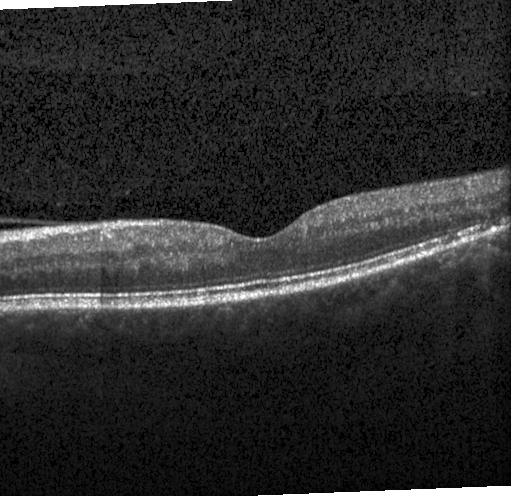
This B-scan demonstrates neither choroidal neovascularization, diabetic macular edema, nor drusen.